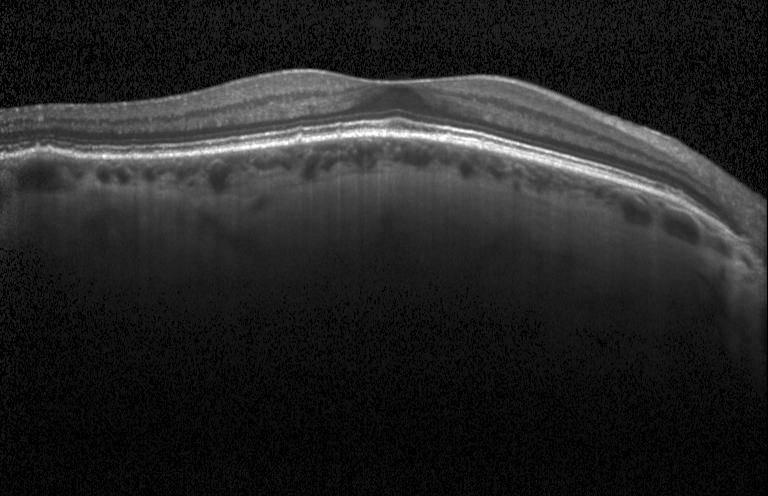

Macular OCT: multiple drusen.